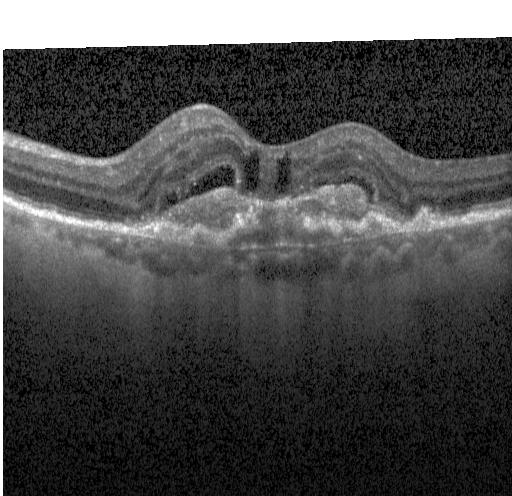
Heidelberg Spectralis. OCT line scan. Macular scan.
Impression: CNV.